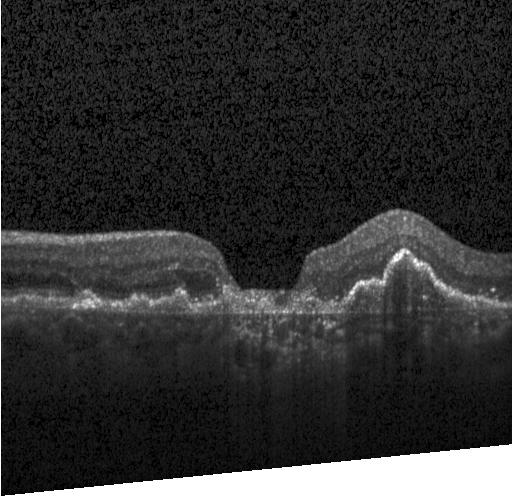 OCT B-scan. Fovea-centered
Impression: a choroidal neovascular membrane.